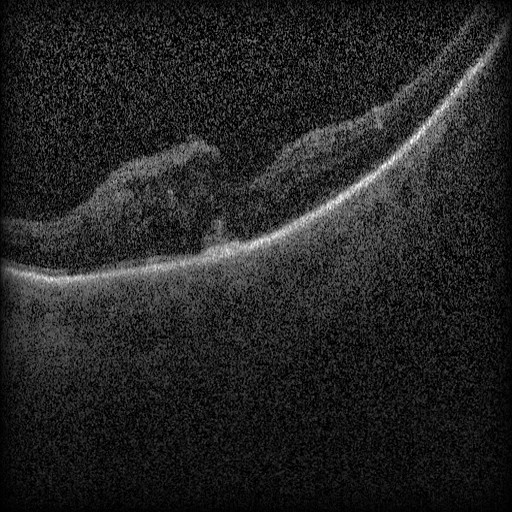 OCT B-scan; through the macula
Finding: diabetic macular edema.